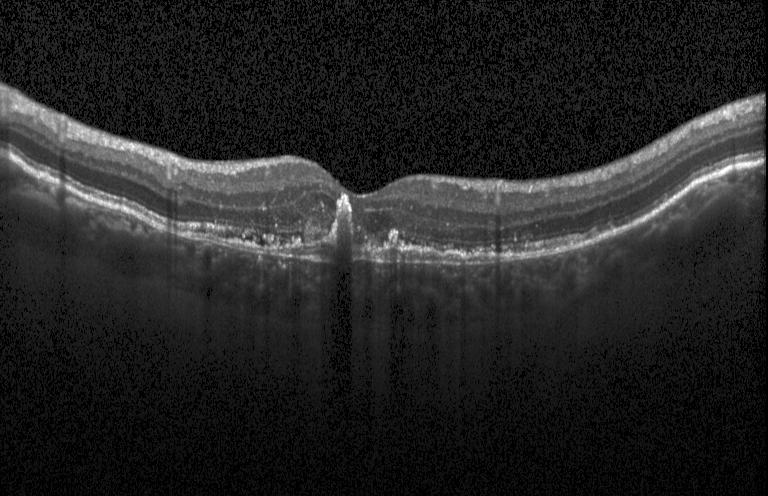 Macular OCT: a choroidal neovascular membrane.